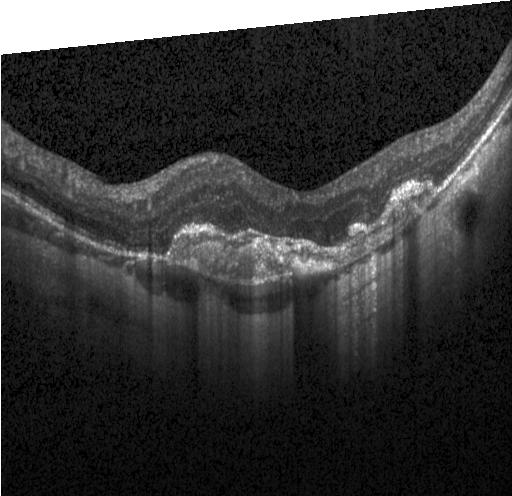
OCT line scan — This B-scan demonstrates choroidal neovascularization (CNV).